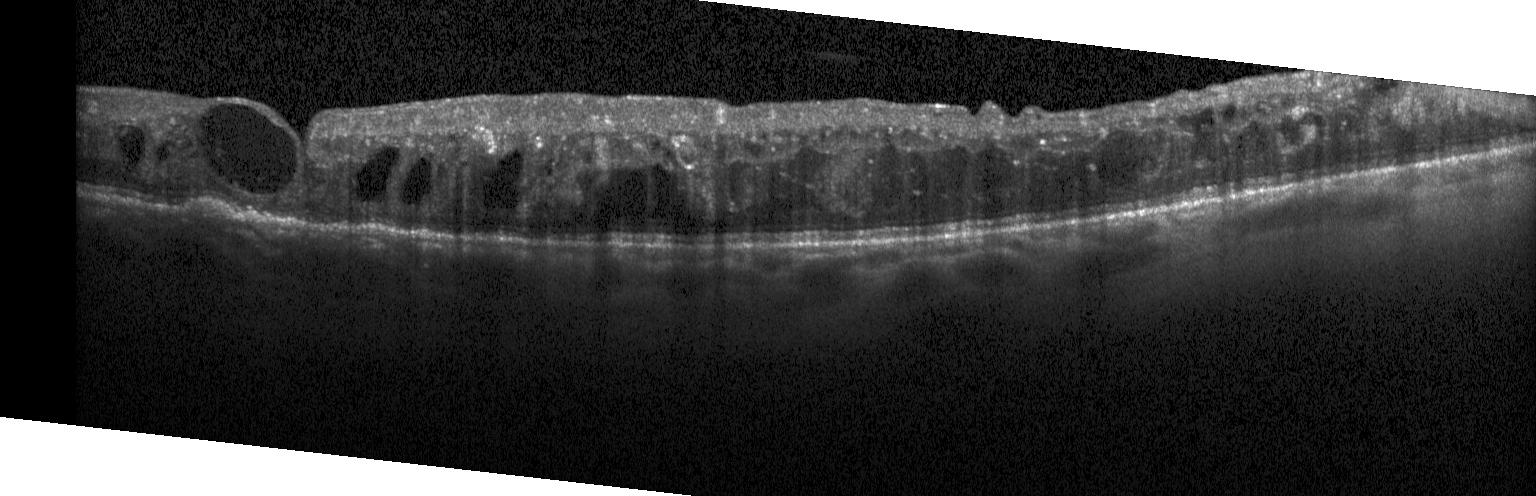
OCT line scan — Diagnosis: diabetic macular edema (DME).